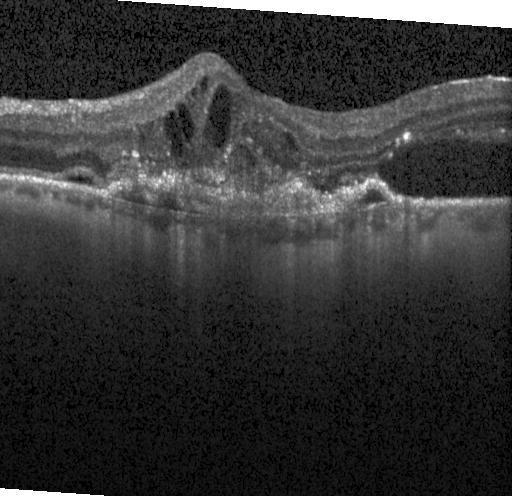 Finding: a choroidal neovascular membrane.